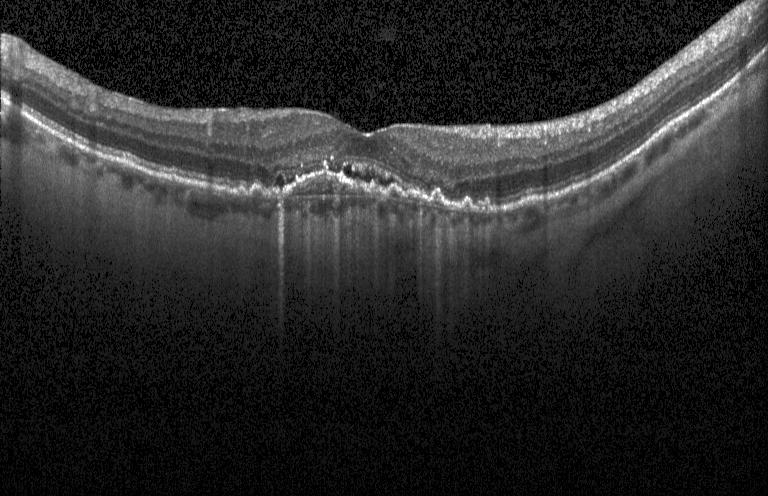
Finding: a choroidal neovascular membrane.